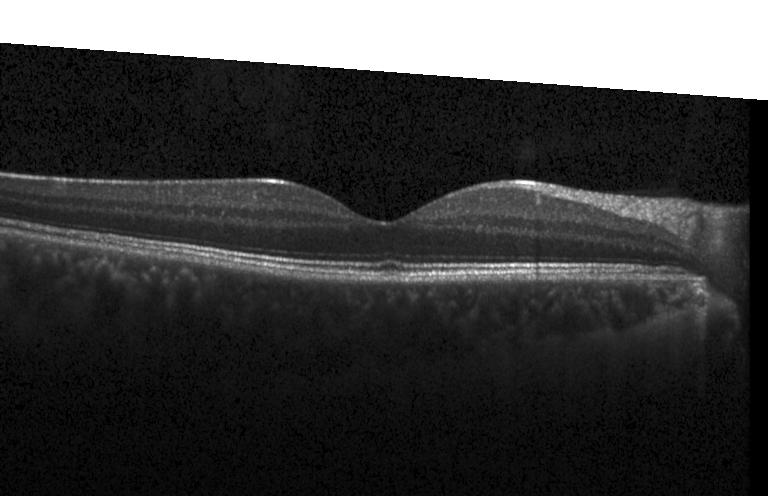

SD-OCT; retinal OCT cross-section; instrument: Heidelberg Spectralis.
Assessment: no choroidal neovascularization, diabetic macular edema, or drusen.